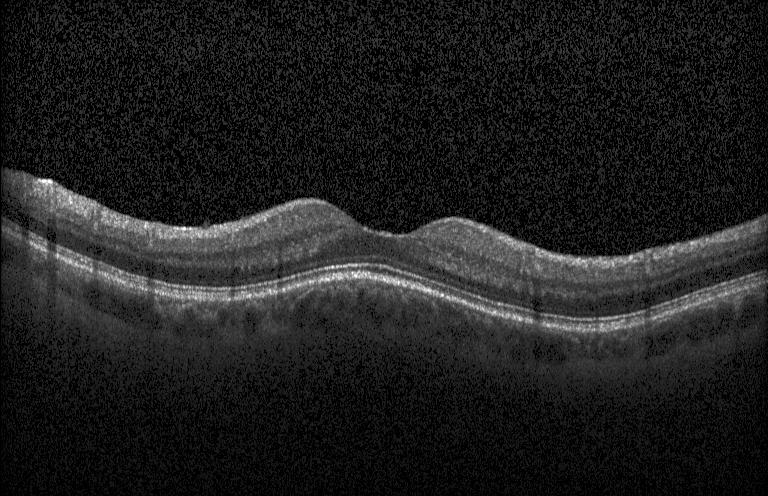
SD-OCT, retinal OCT B-scan, acquired on a Heidelberg Spectralis — Impression: no choroidal neovascularization, diabetic macular edema, or drusen.